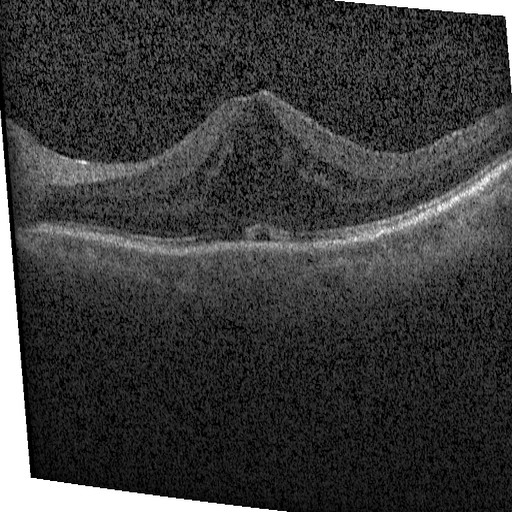 The scan shows diabetic macular edema.